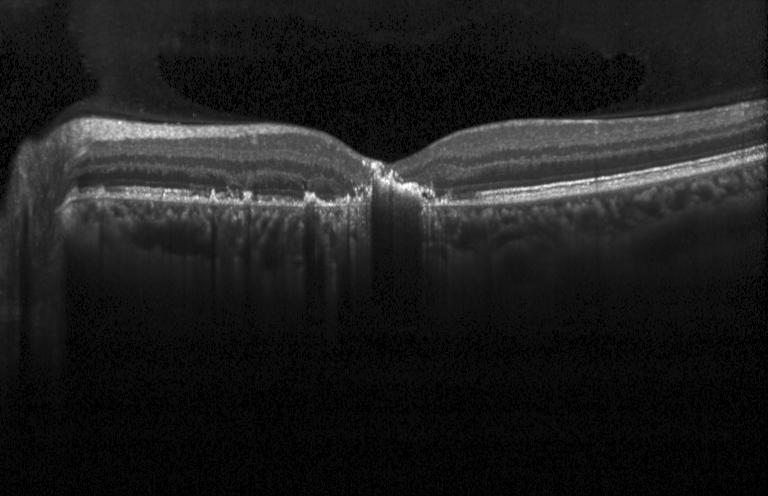 OCT B-scan — Macular OCT: choroidal neovascularization.